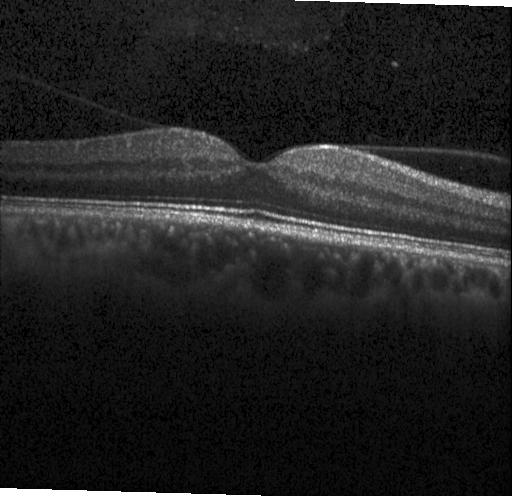 Retinal OCT B-scan · spectral-domain OCT · horizontal scan through the fovea · Heidelberg Spectralis OCT system
Impression: no choroidal neovascularization, diabetic macular edema, or drusen.